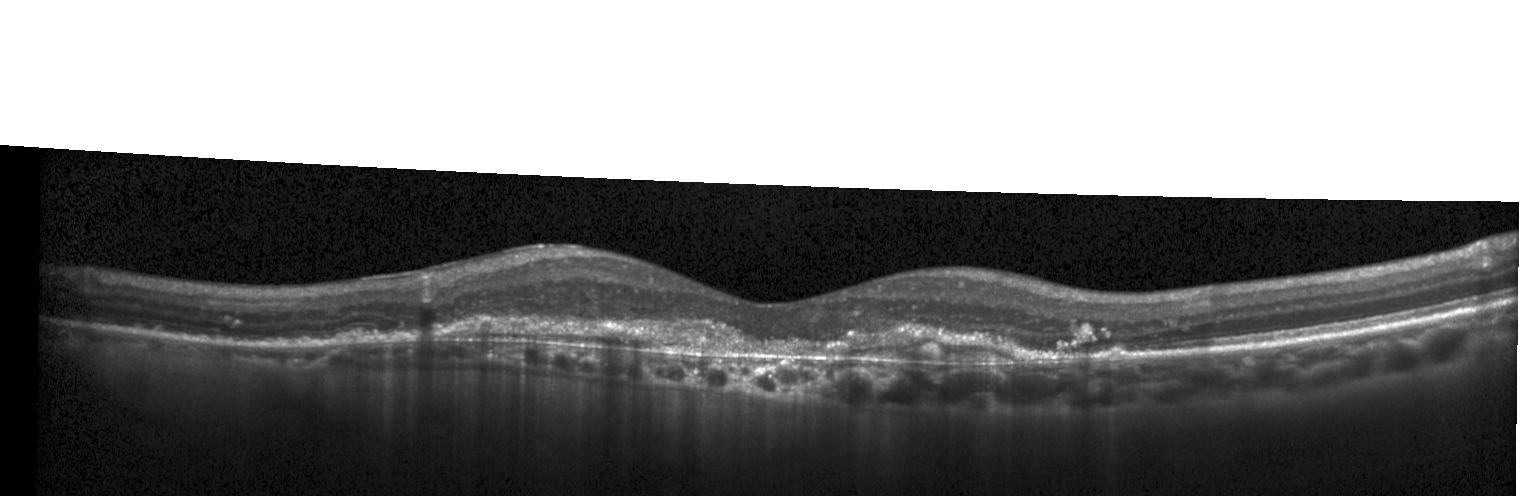 This B-scan demonstrates a choroidal neovascular membrane.